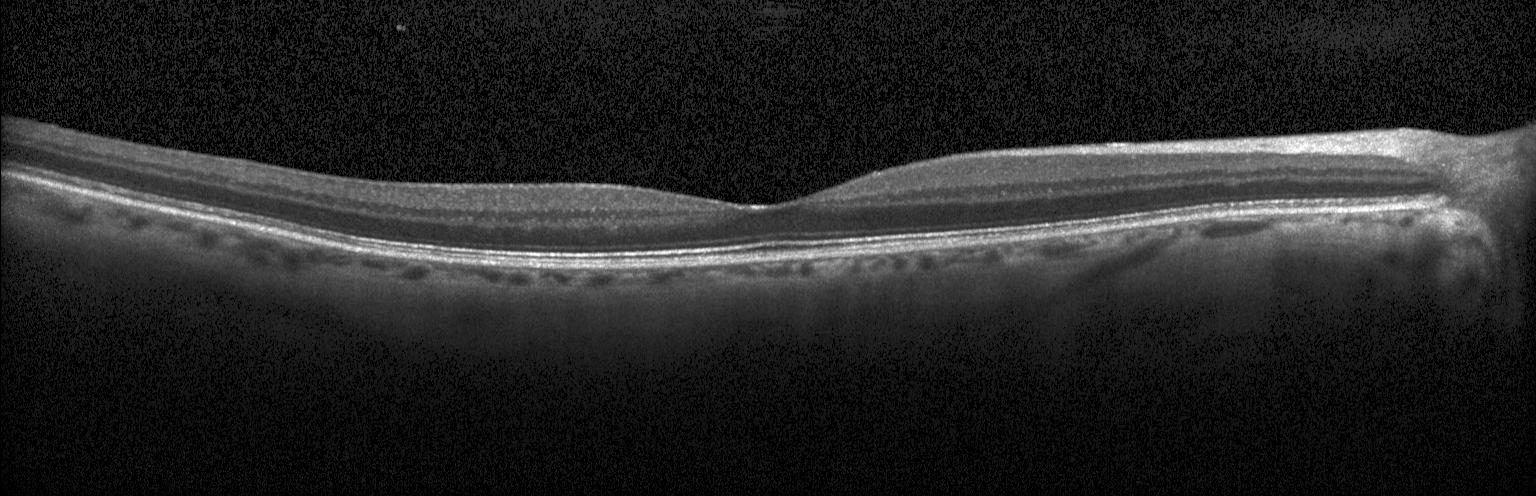

OCT B-scan. No CNV, DME, or drusen.